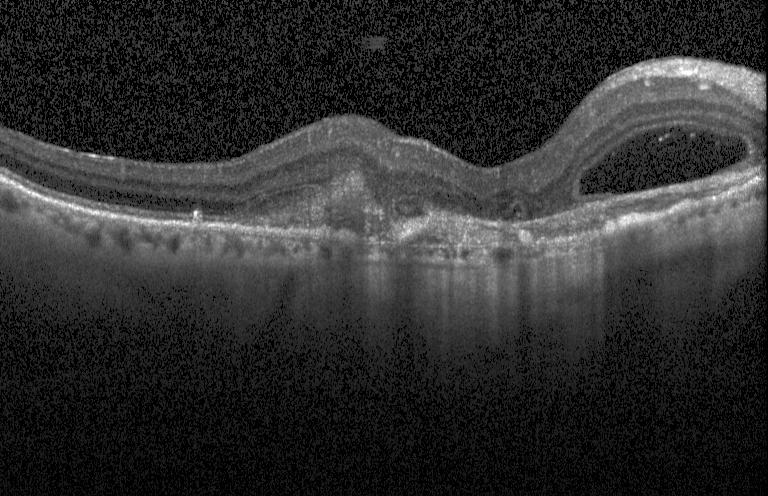
Retinal OCT B-scan — Macular OCT: CNV.